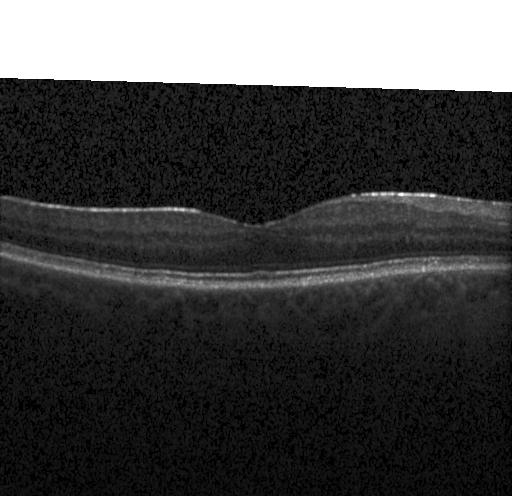
Heidelberg Spectralis OCT system, macular scan, spectral-domain optical coherence tomography, retinal OCT B-scan.
Macular OCT: neither choroidal neovascularization, diabetic macular edema, nor drusen.